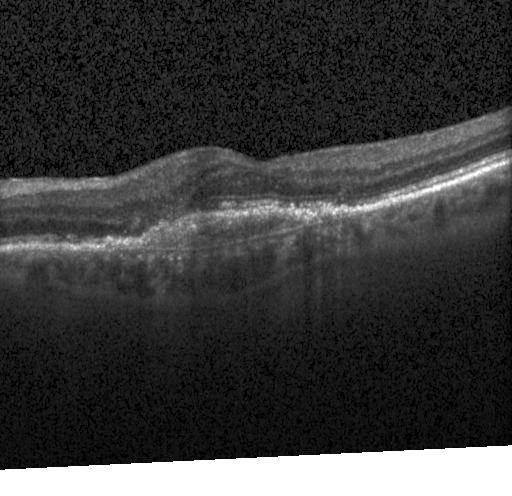
Diagnosis: a choroidal neovascular membrane.